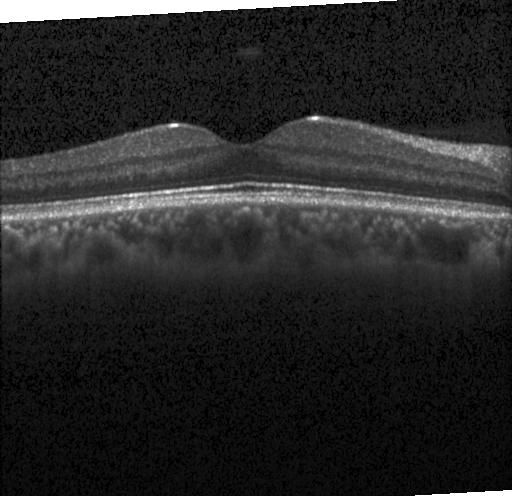
Acquired on a Heidelberg Spectralis · through the macula · SD-OCT · OCT line scan
No choroidal neovascularization, no diabetic macular edema, and no drusen.